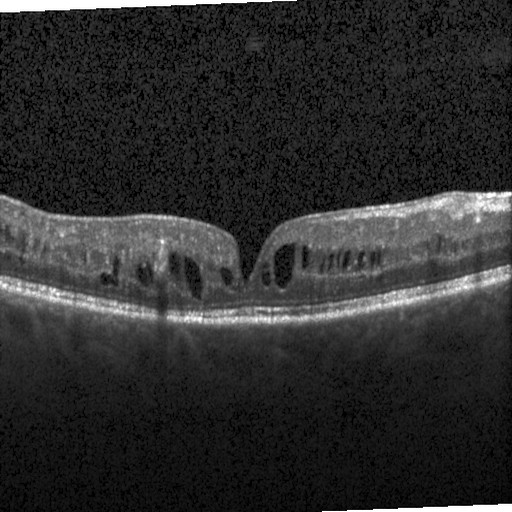

Macular OCT: diabetic macular edema (DME).